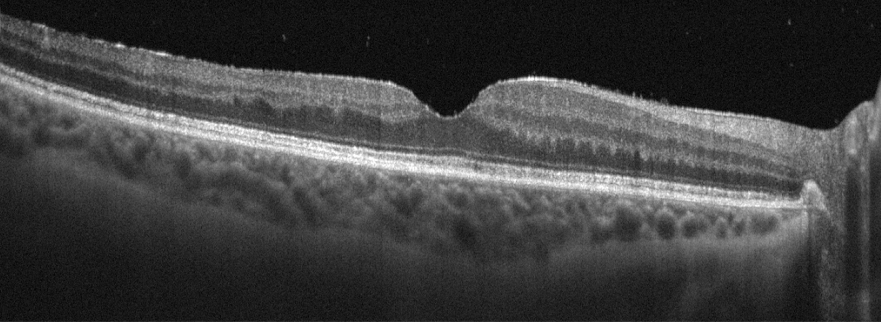 Assessment: epiretinal membrane.